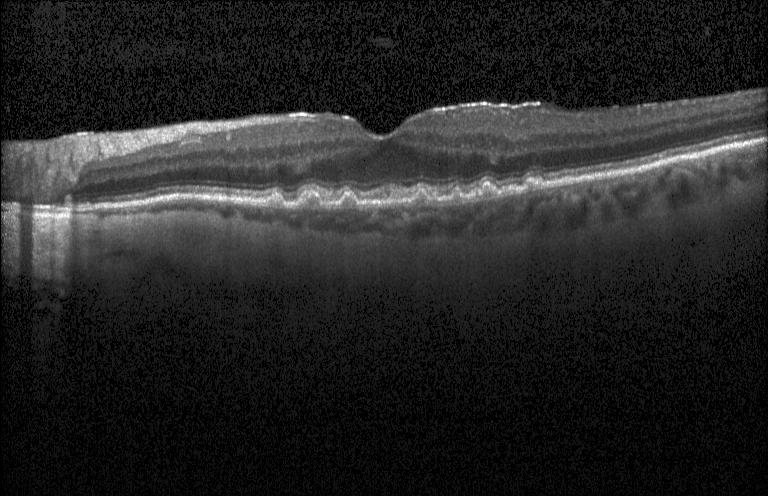 Spectral-domain OCT B-scan: drusen.